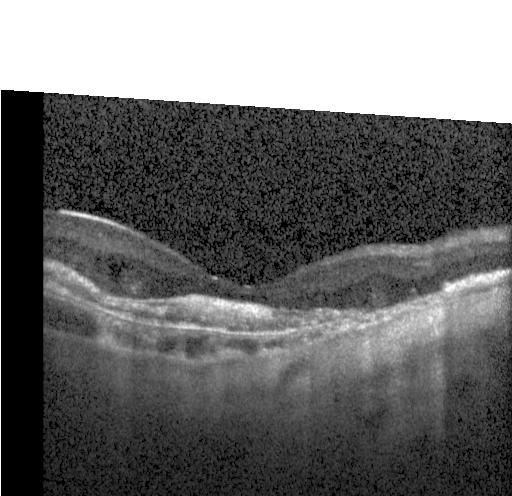 Optical coherence tomography scan
Diagnosis: a choroidal neovascular membrane.